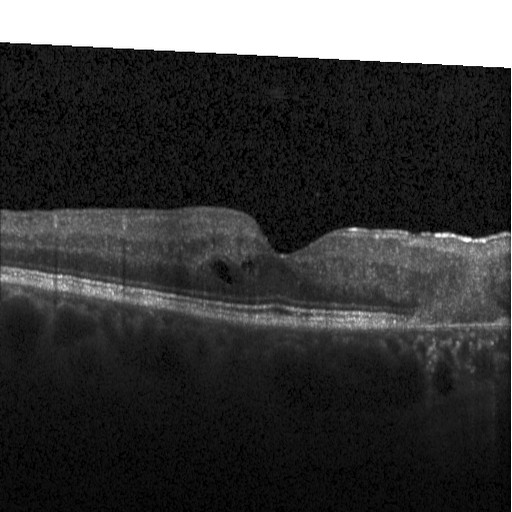

Finding: DME.